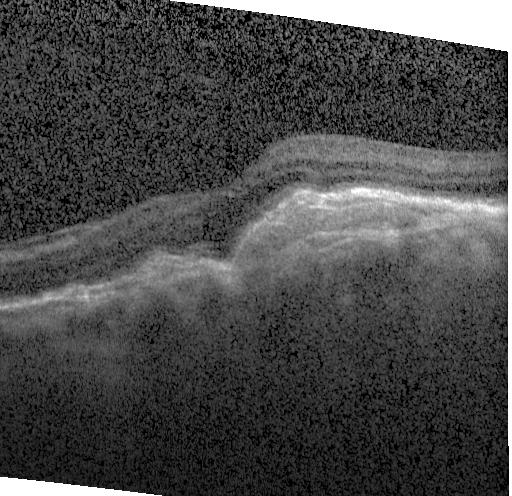
Retinal OCT B-scan
Assessment: choroidal neovascularization.